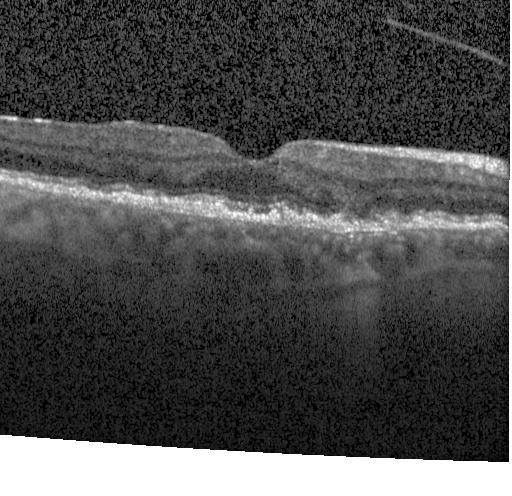

Finding: sub-RPE drusenoid deposits.